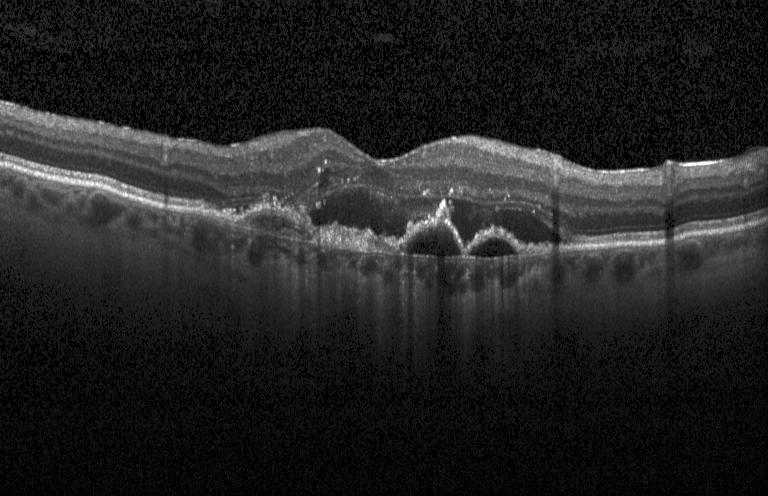
OCT B-scan.
Diagnosis: a choroidal neovascular membrane.